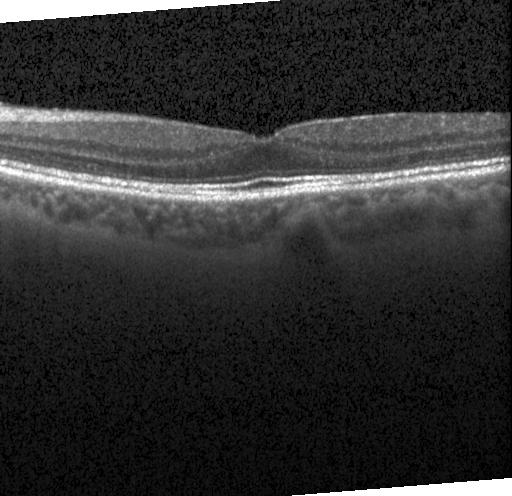 Spectral-domain optical coherence tomography · Heidelberg Spectralis · retinal OCT cross-section · fovea-centered.
Finding: no evidence of choroidal neovascularization, diabetic macular edema, or drusen.